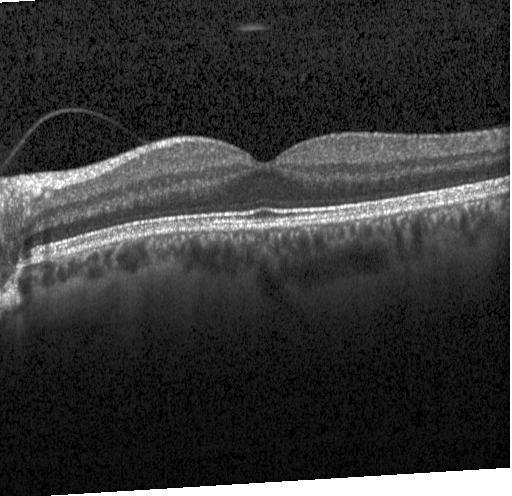

Diagnosis: neither CNV, DME, nor drusen.